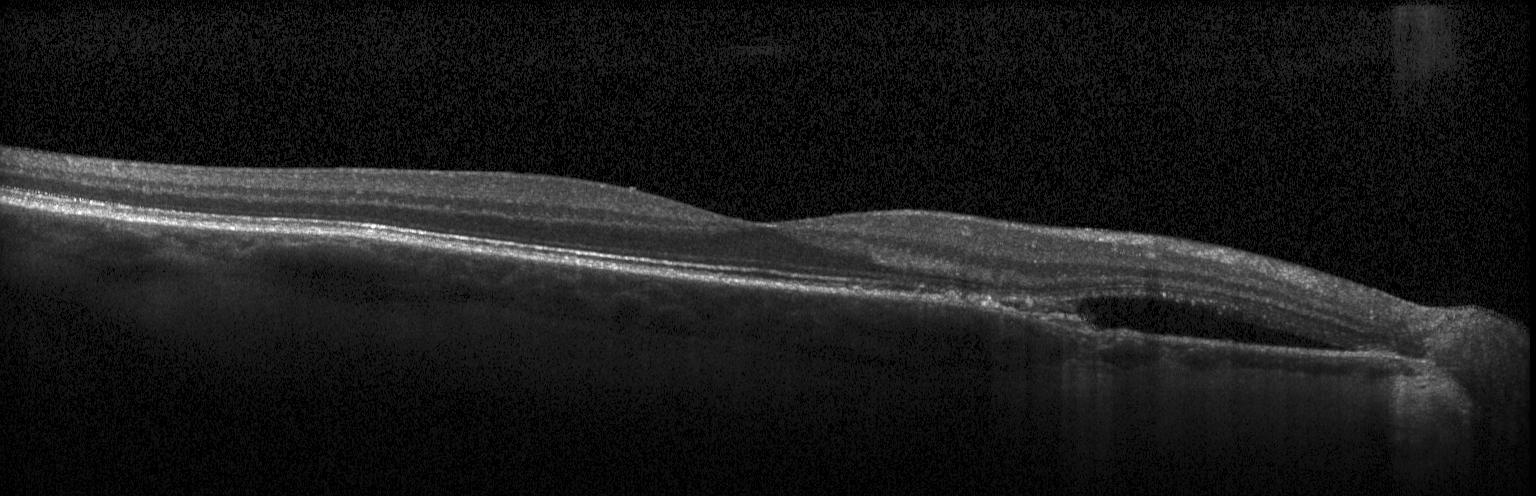
Retinal OCT cross-section showing choroidal neovascularization.